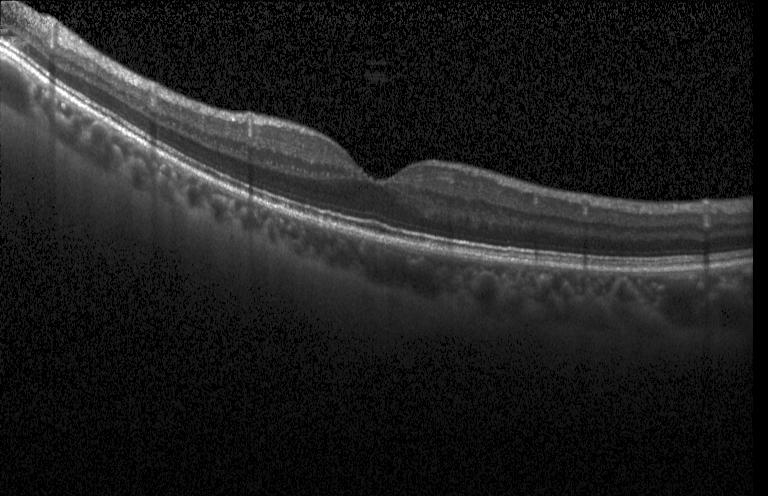 Diagnosis: no CNV, DME, or drusen.